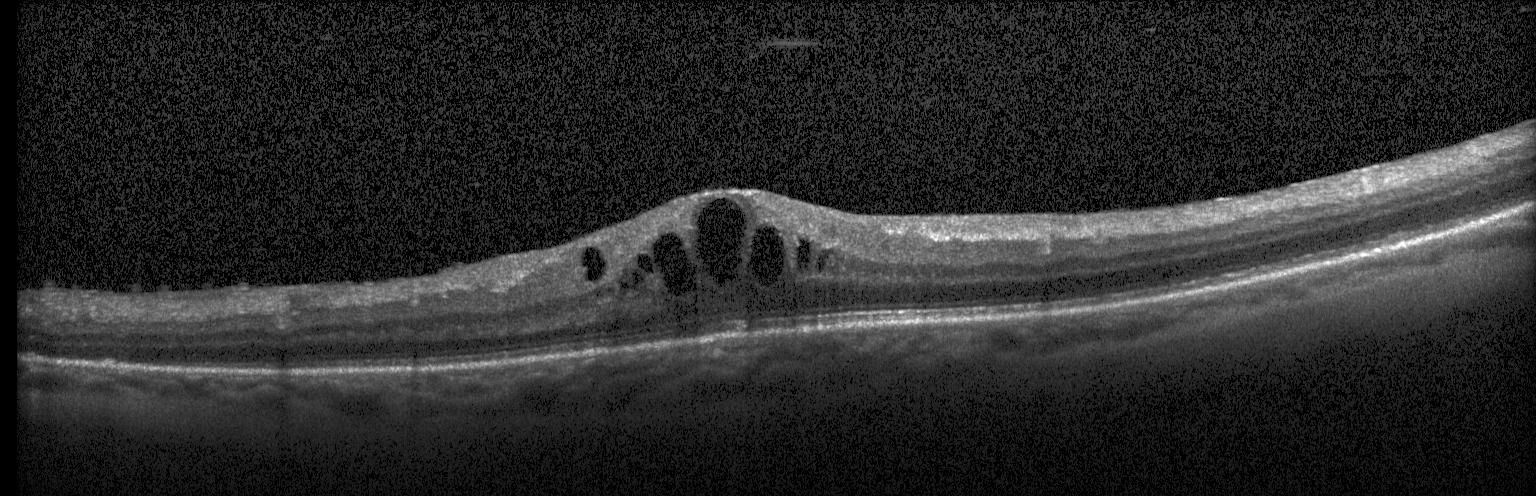
Retinal OCT cross-section showing diabetic macular edema.